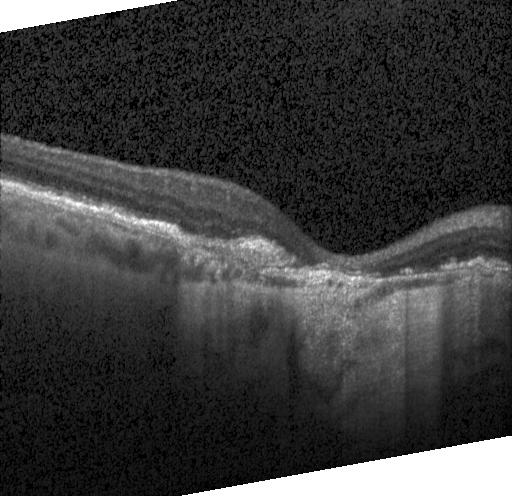
Retinal OCT B-scan · instrument: Heidelberg Spectralis · macular scan
The scan shows CNV.